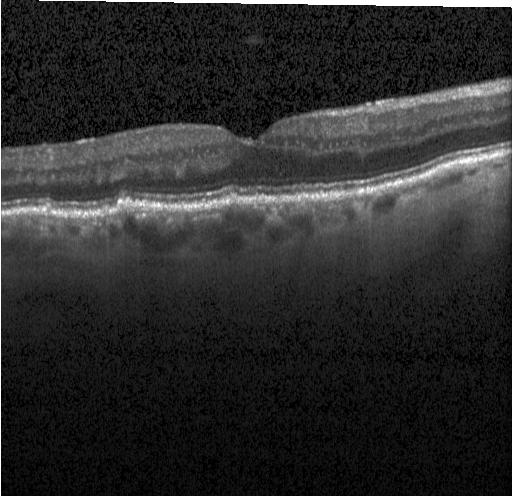

This B-scan demonstrates sub-RPE drusenoid deposits.